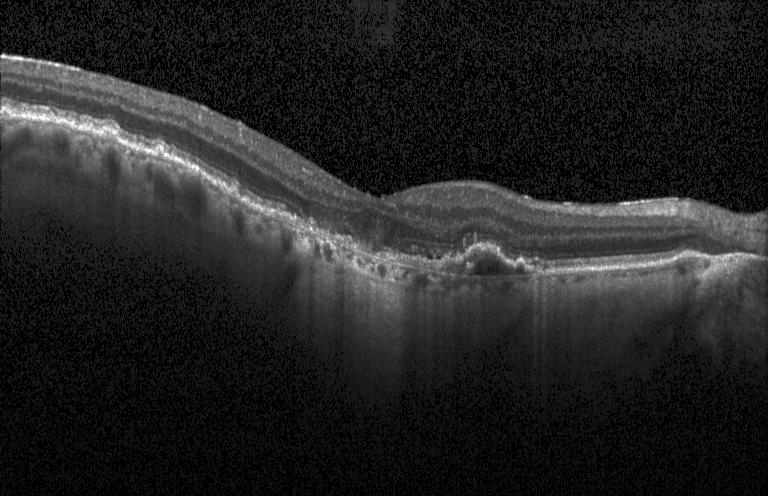 OCT finding: a choroidal neovascular membrane.